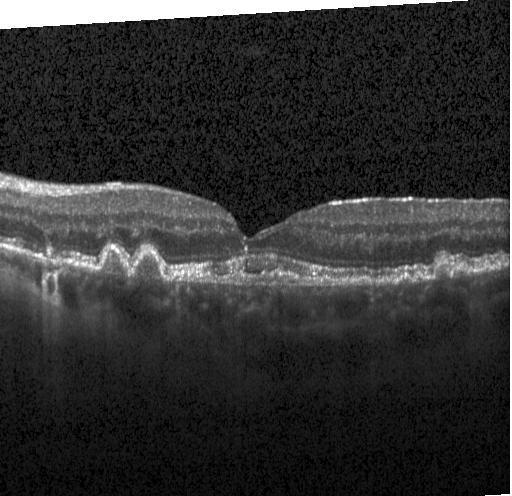

Optical coherence tomography B-scan, instrument: Heidelberg Spectralis, spectral-domain optical coherence tomography.
Dx: CNV.